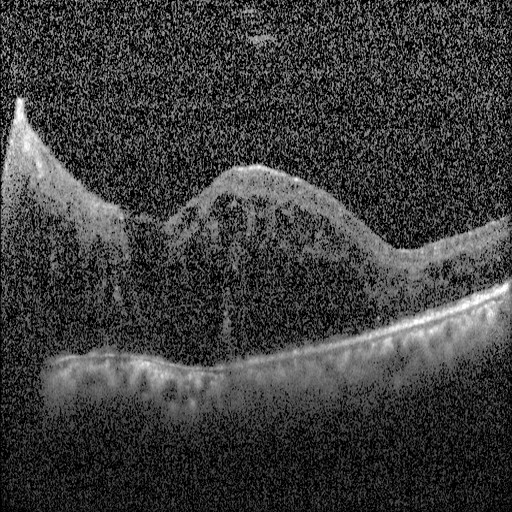 Heidelberg Spectralis OCT system · spectral-domain optical coherence tomography · retinal OCT B-scan · centered on the fovea. This B-scan demonstrates diabetic macular edema (DME).